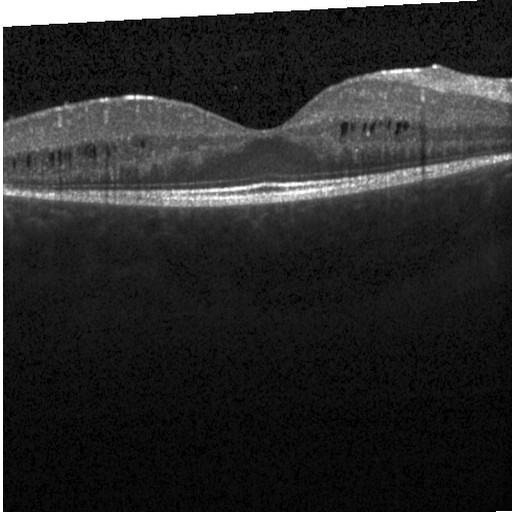
The scan shows DME.